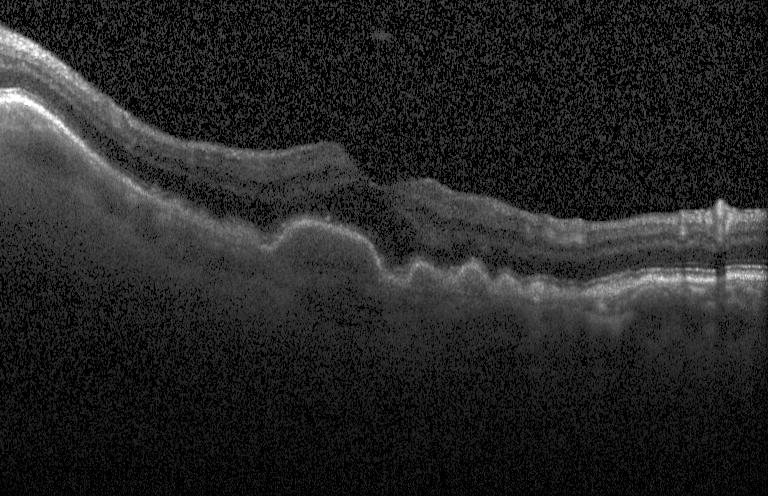

Retinal OCT B-scan — Diagnosis: drusen.